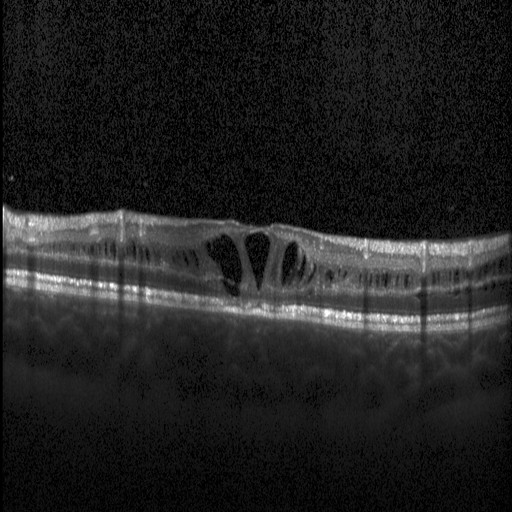 Centered on the fovea; OCT line scan — Diagnosis: DME.